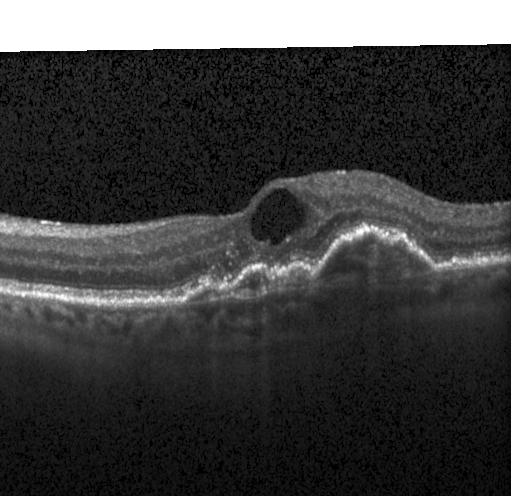
Spectral-domain optical coherence tomography. Heidelberg Spectralis. OCT B-scan. This B-scan demonstrates choroidal neovascularization.